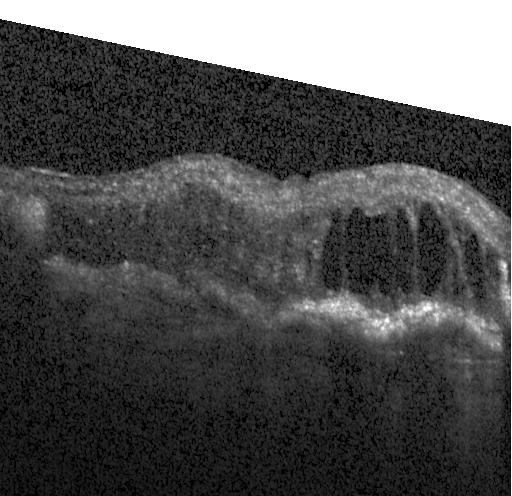
Centered on the fovea, retinal OCT cross-section
Finding: a choroidal neovascular membrane.